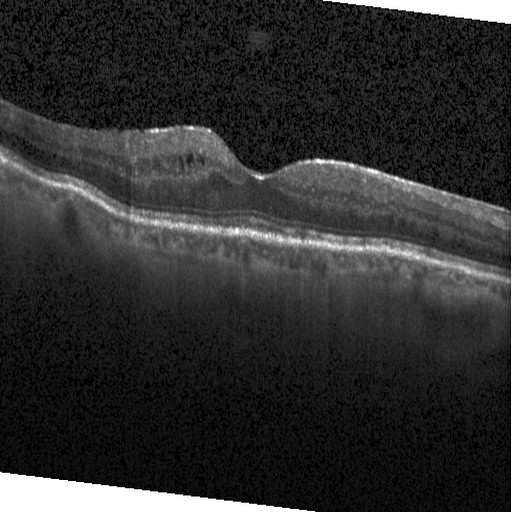
Optical coherence tomography B-scan — Finding: diabetic macular edema (DME).